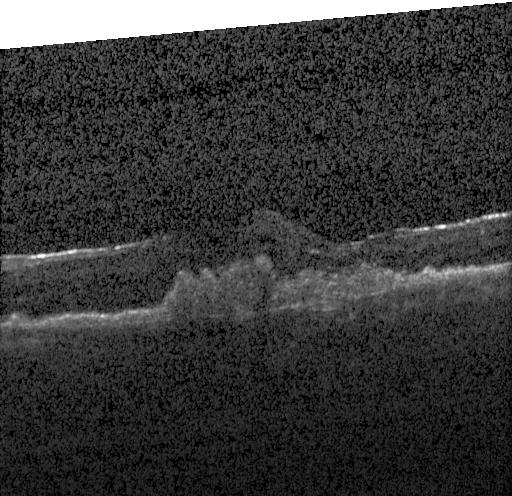

Centered on the fovea, SD-OCT, OCT line scan, acquired on a Heidelberg Spectralis. OCT finding: a choroidal neovascular membrane.